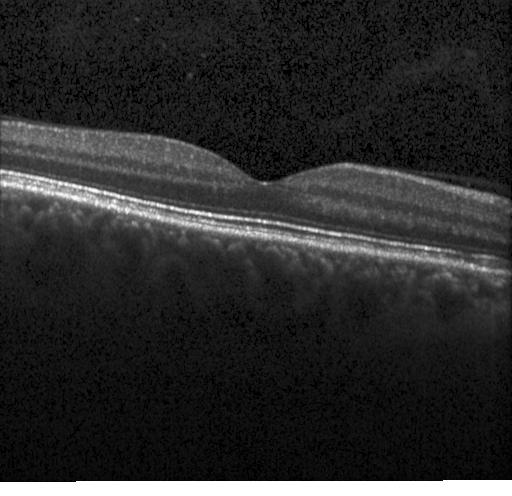
OCT B-scan.
Macular OCT: no evidence of choroidal neovascularization, diabetic macular edema, or drusen.